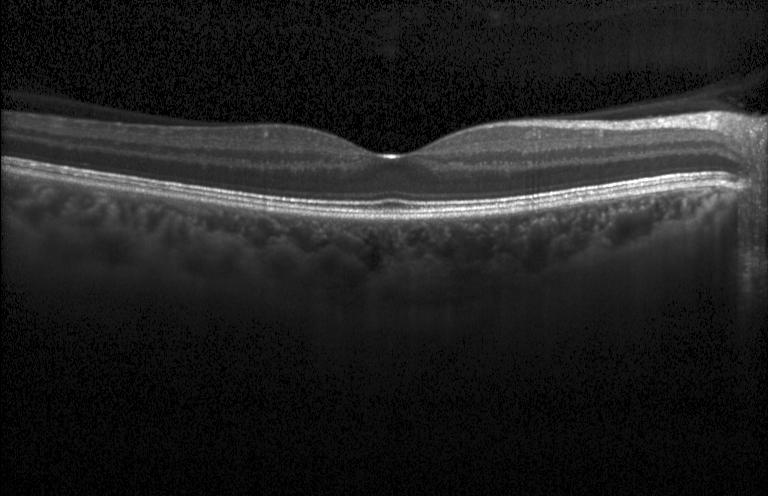
Optical coherence tomography B-scan · spectral-domain optical coherence tomography — OCT finding: no CNV, DME, or drusen.